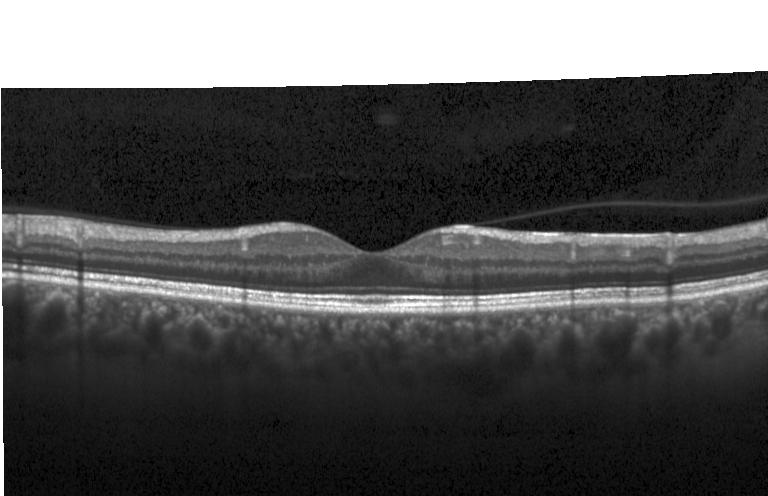

SD-OCT, macular scan, retinal OCT cross-section
Dx: no evidence of CNV, DME, or drusen.